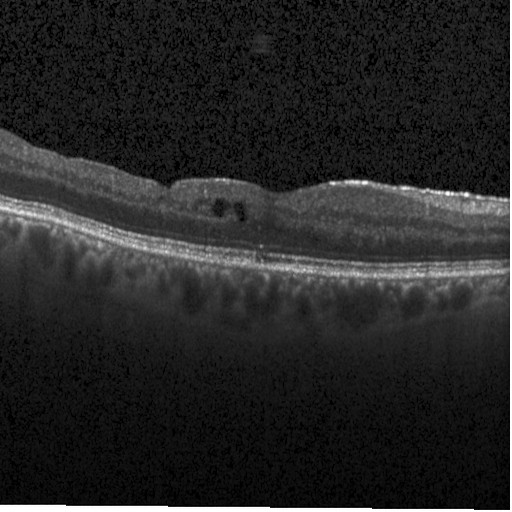
OCT B-scan. Impression: diabetic macular edema.